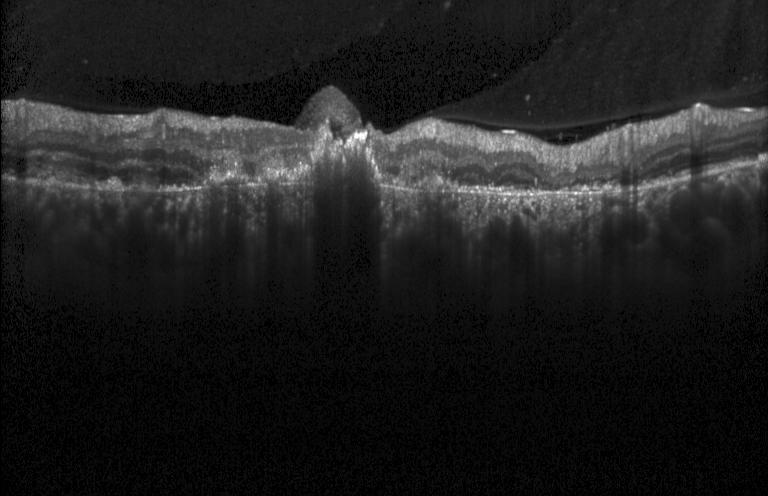 Macular scan · OCT B-scan. Diagnosis: a choroidal neovascular membrane.